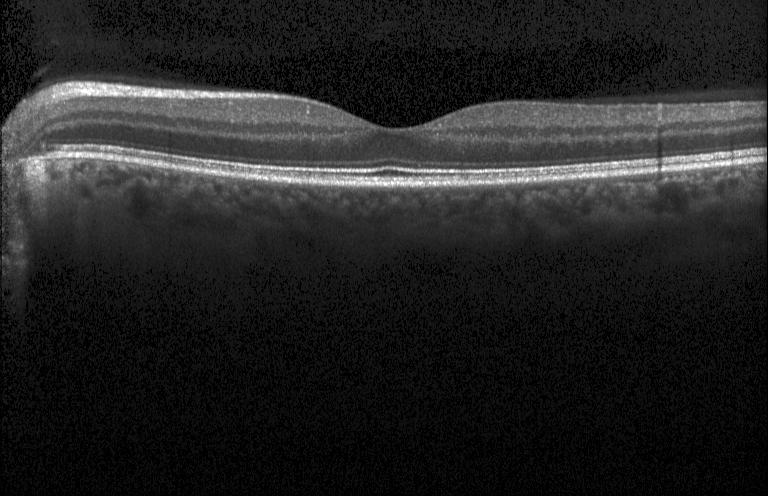

Heidelberg Spectralis OCT system · optical coherence tomography scan · macular scan · spectral-domain OCT. Finding: no choroidal neovascularization, no diabetic macular edema, and no drusen.